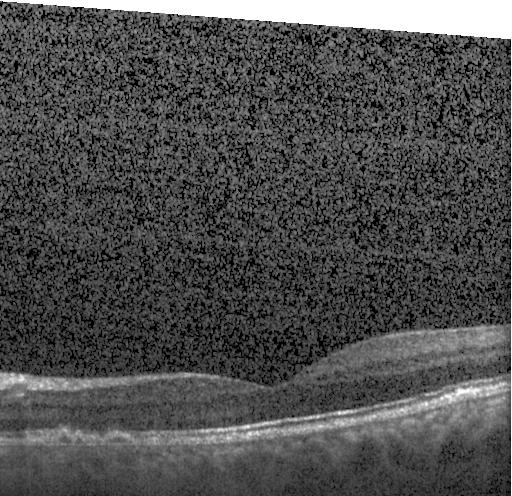
OCT line scan — Impression: a choroidal neovascular membrane.